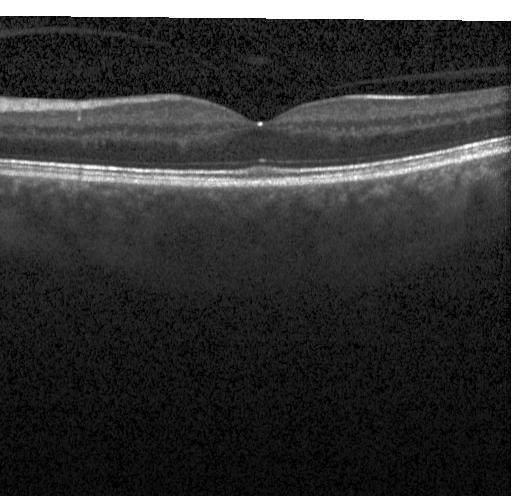

Diagnosis: no evidence of CNV, DME, or drusen.